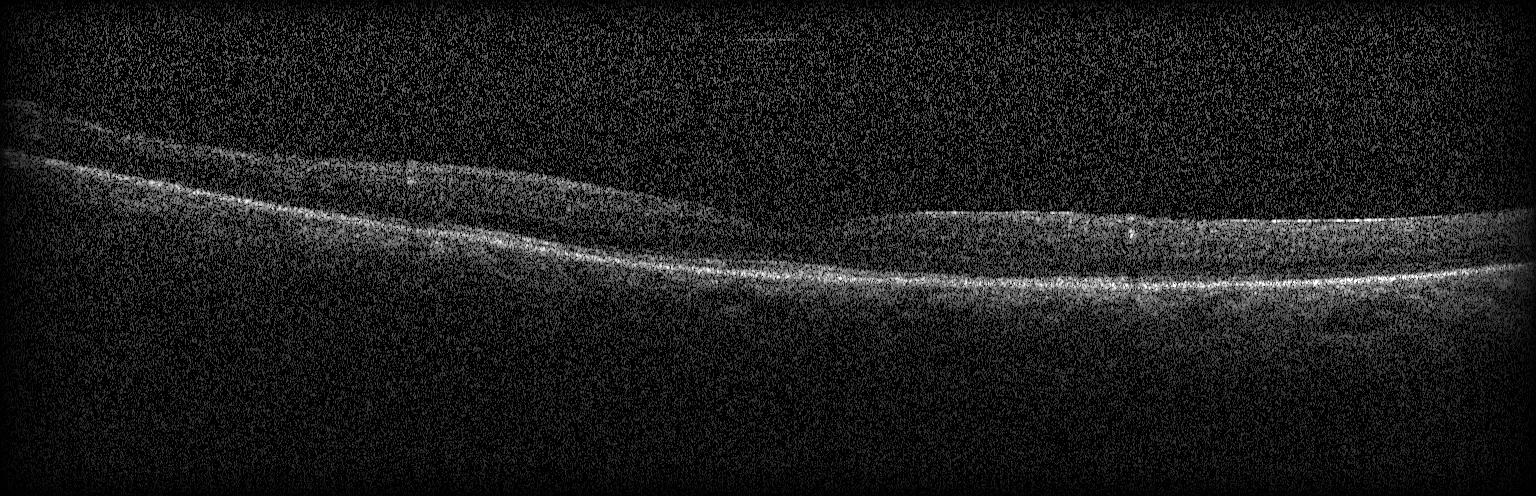

Retinal OCT cross-section · spectral-domain OCT.
Diagnosis: no choroidal neovascularization, diabetic macular edema, or drusen.